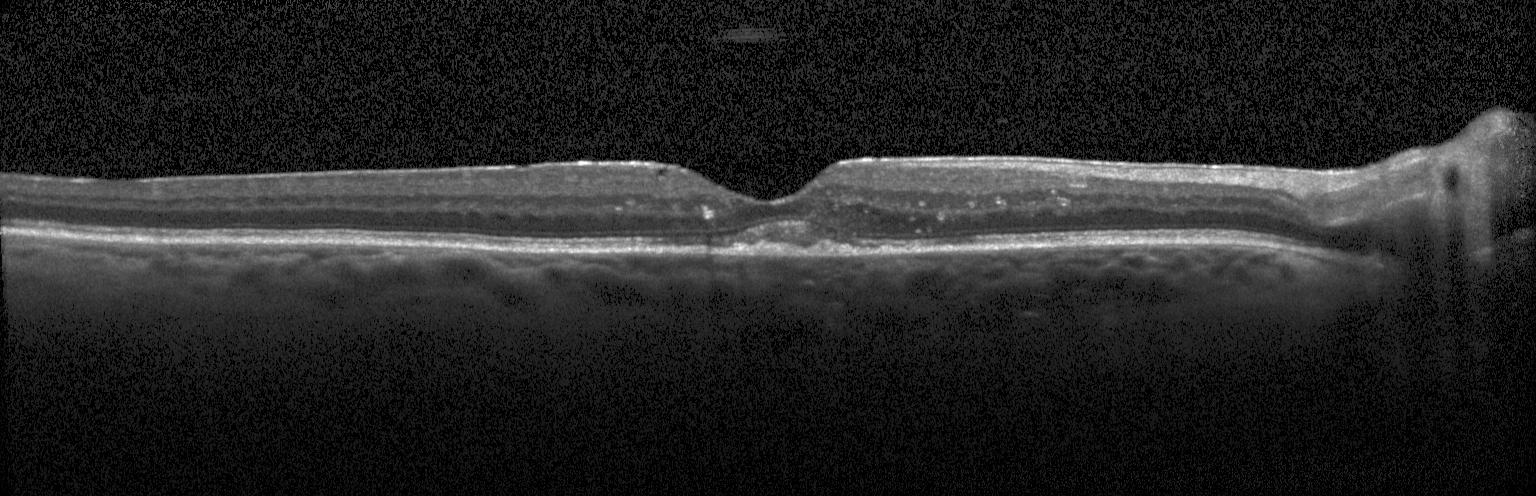

Acquired on a Heidelberg Spectralis · retinal OCT cross-section · spectral-domain OCT.
Diagnosis: a choroidal neovascular membrane.